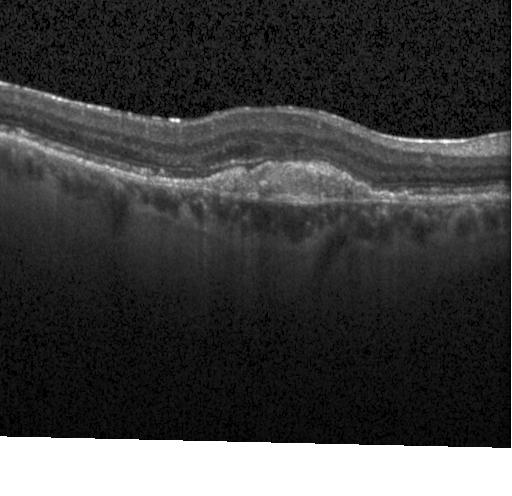

Optical coherence tomography scan — Finding: choroidal neovascularization (CNV).